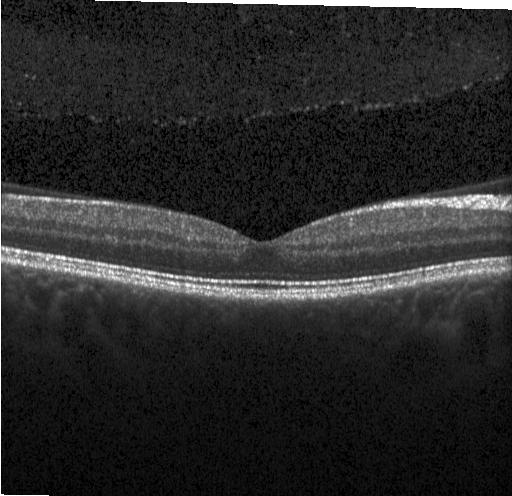
Fovea-centered; OCT B-scan. Diagnosis: no evidence of CNV, DME, or drusen.